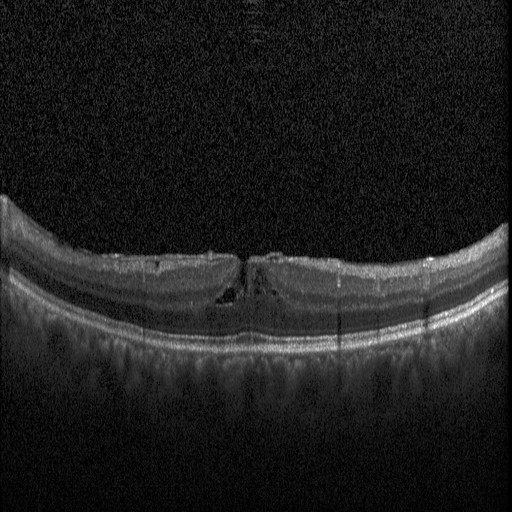 Centered on the fovea · retinal OCT cross-section.
Assessment: diabetic macular edema (DME).